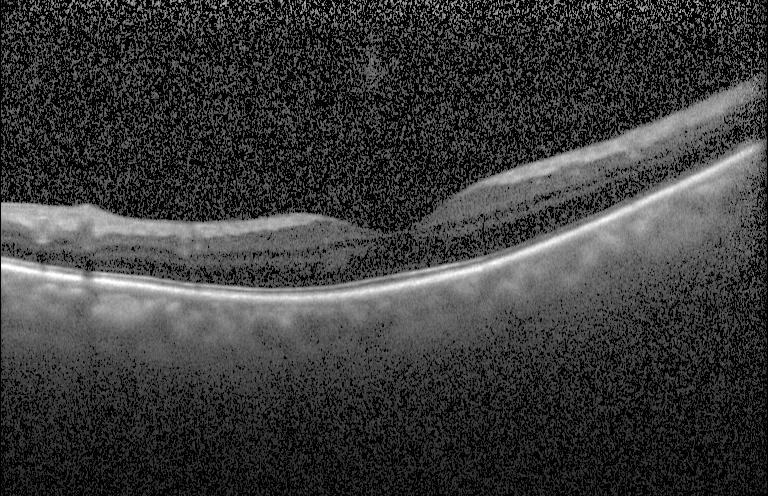 Impression: no evidence of CNV, DME, or drusen.